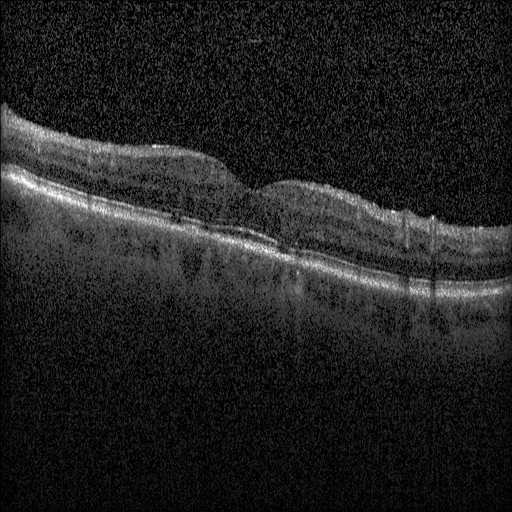

Centered on the fovea. Spectral-domain optical coherence tomography. Retinal OCT cross-section. Finding: diabetic macular edema (DME).